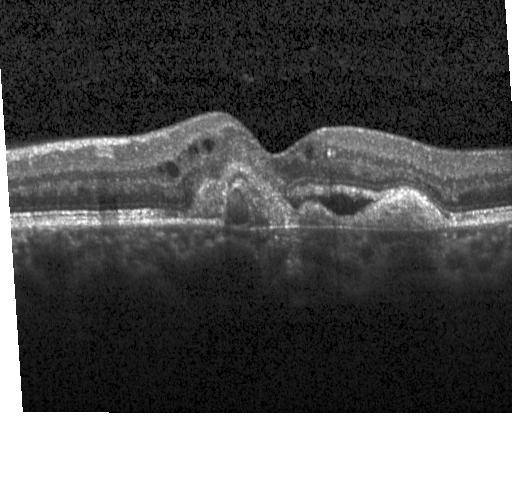
Optical coherence tomography scan; fovea-centered; spectral-domain optical coherence tomography.
Finding: choroidal neovascularization.